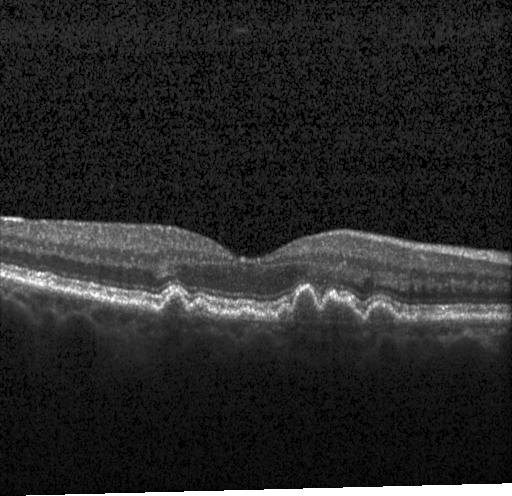 SD-OCT · optical coherence tomography scan · Heidelberg Spectralis
Assessment: multiple drusen.